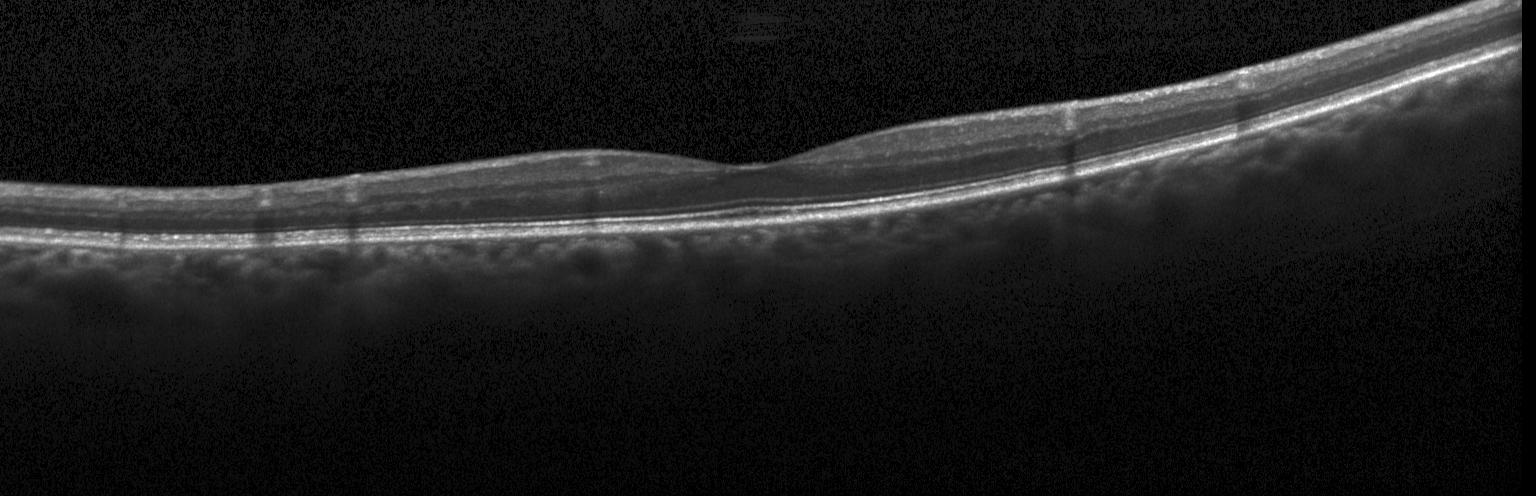
Through the macula. Heidelberg Spectralis OCT system. Spectral-domain optical coherence tomography. Retinal OCT cross-section.
This B-scan demonstrates no choroidal neovascularization, no diabetic macular edema, and no drusen.